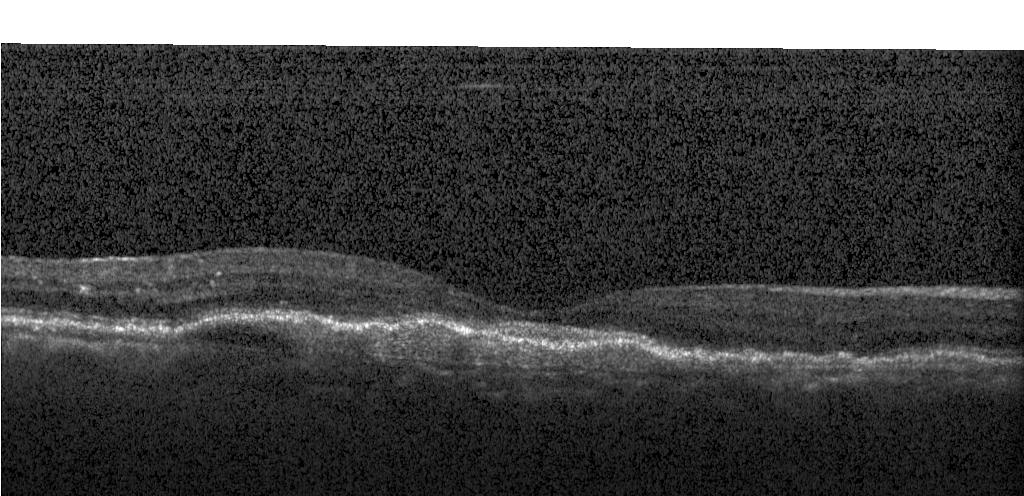

Optical coherence tomography B-scan. OCT finding: choroidal neovascularization.